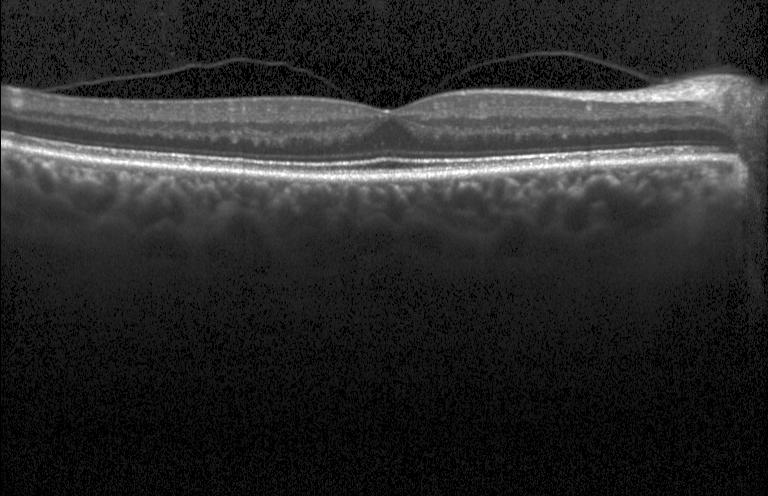
OCT line scan, spectral-domain optical coherence tomography, instrument: Heidelberg Spectralis, horizontal scan through the fovea — Finding: neither choroidal neovascularization, diabetic macular edema, nor drusen.